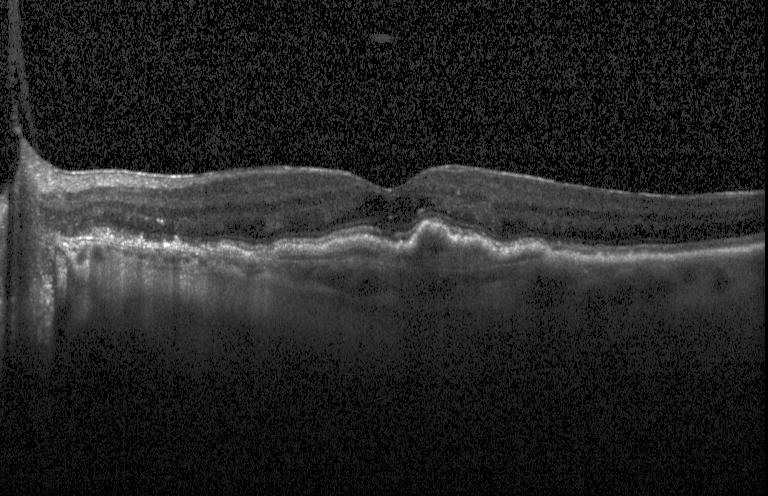

Acquired on a Heidelberg Spectralis, horizontal scan through the fovea, optical coherence tomography scan. The scan shows CNV.